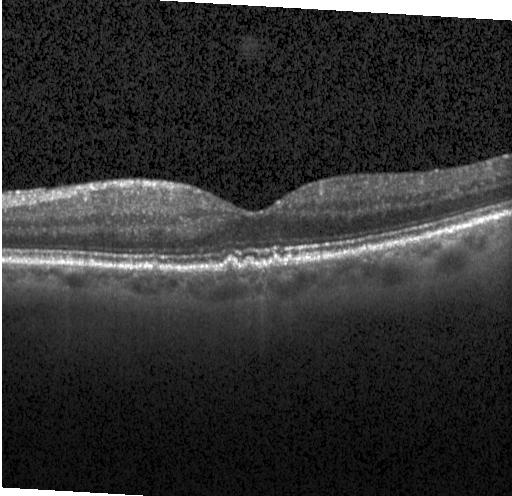 Impression: sub-RPE drusenoid deposits.